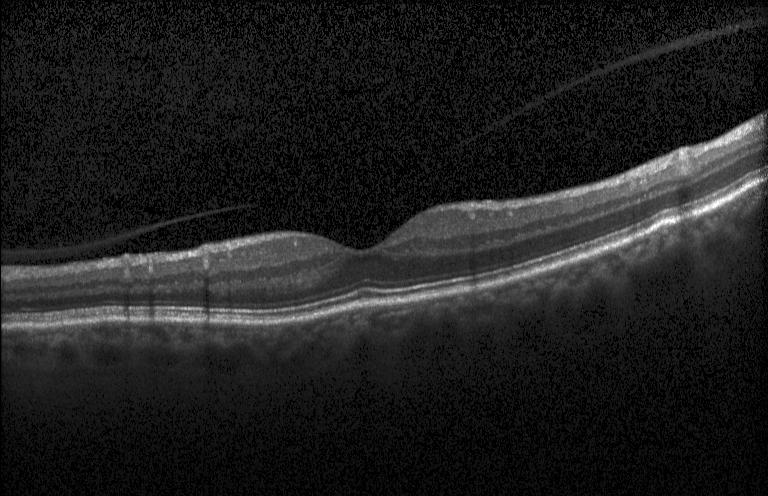
Optical coherence tomography B-scan. This B-scan demonstrates no choroidal neovascularization, diabetic macular edema, or drusen.